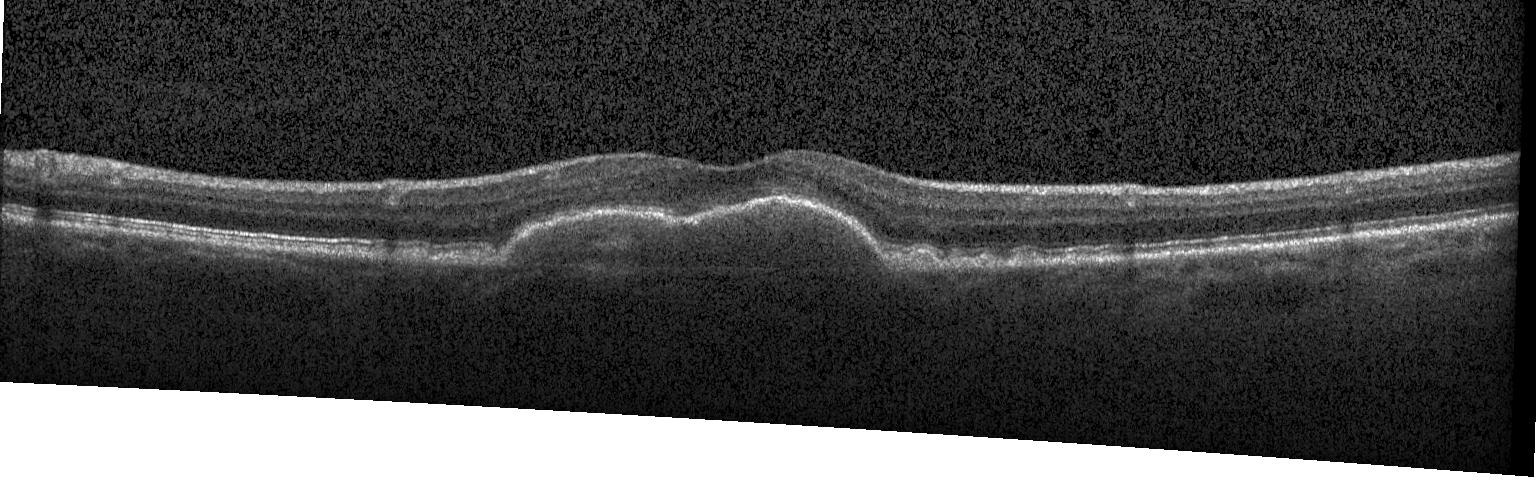
OCT line scan · SD-OCT.
Macular OCT: a choroidal neovascular membrane.